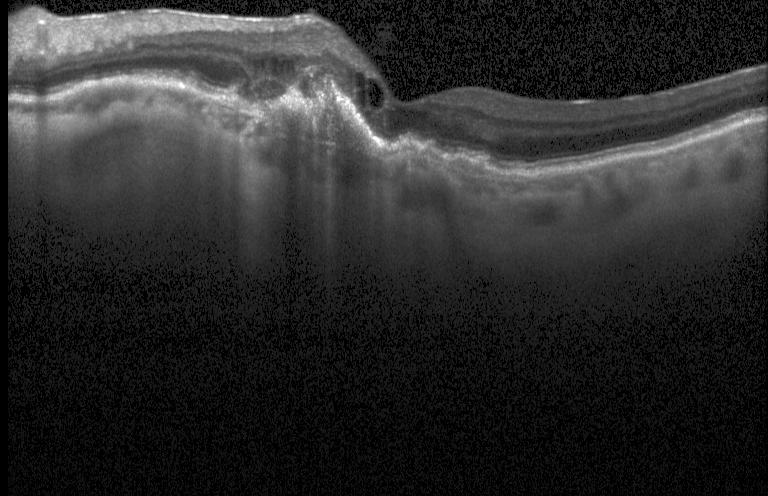

Impression: choroidal neovascularization (CNV).